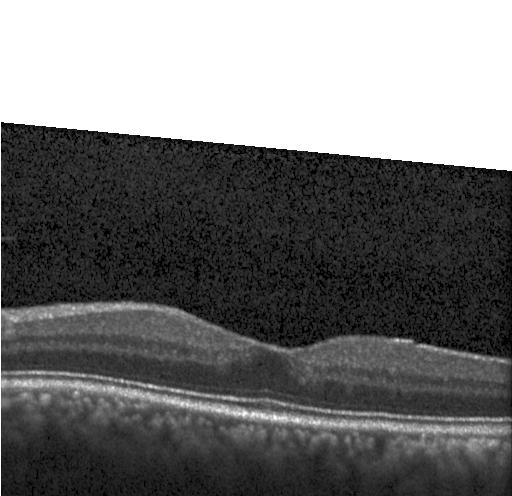
SD-OCT. Heidelberg Spectralis OCT system. Centered on the fovea. OCT B-scan.
OCT finding: neither choroidal neovascularization, diabetic macular edema, nor drusen.